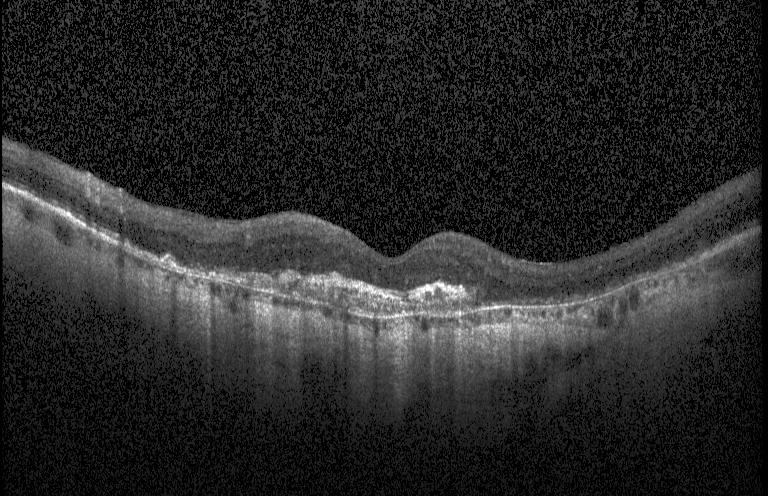 Retinal OCT B-scan. OCT finding: a choroidal neovascular membrane.